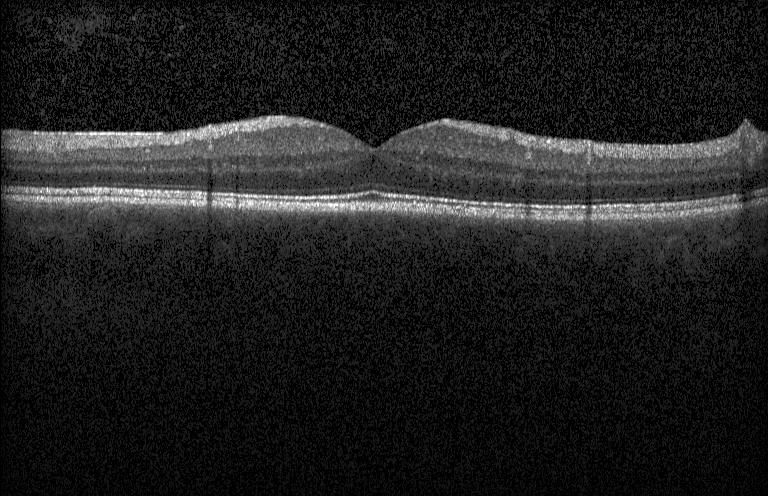 Assessment: no choroidal neovascularization, diabetic macular edema, or drusen.